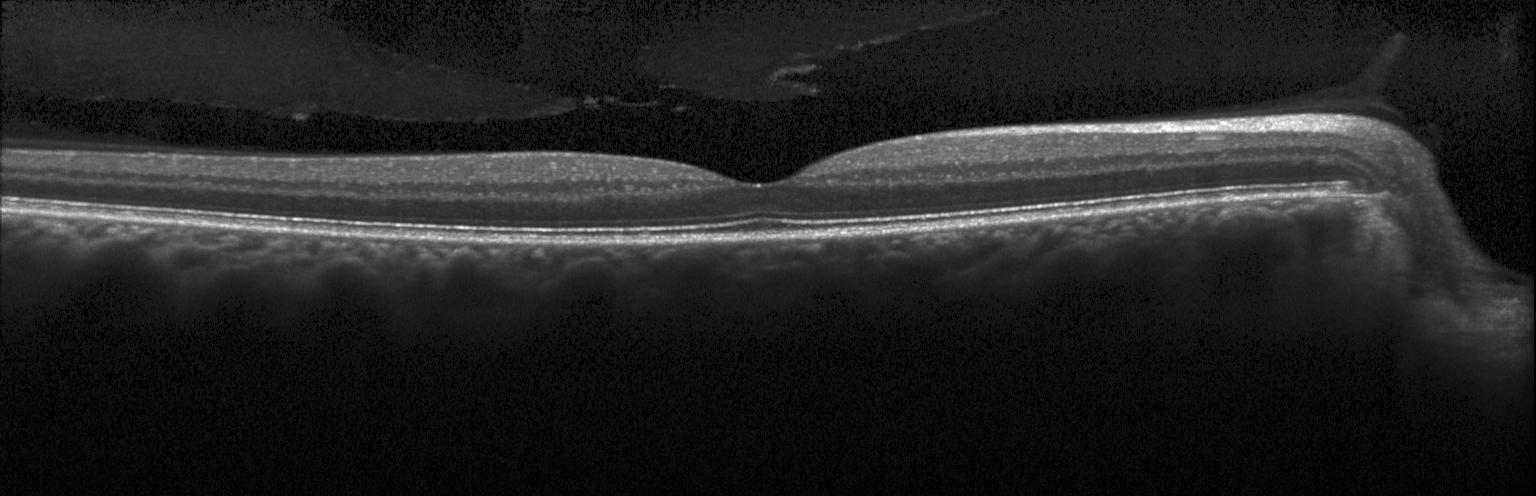

Optical coherence tomography scan. SD-OCT. Instrument: Heidelberg Spectralis. Horizontal scan through the fovea — Macular OCT: no choroidal neovascularization, no diabetic macular edema, and no drusen.